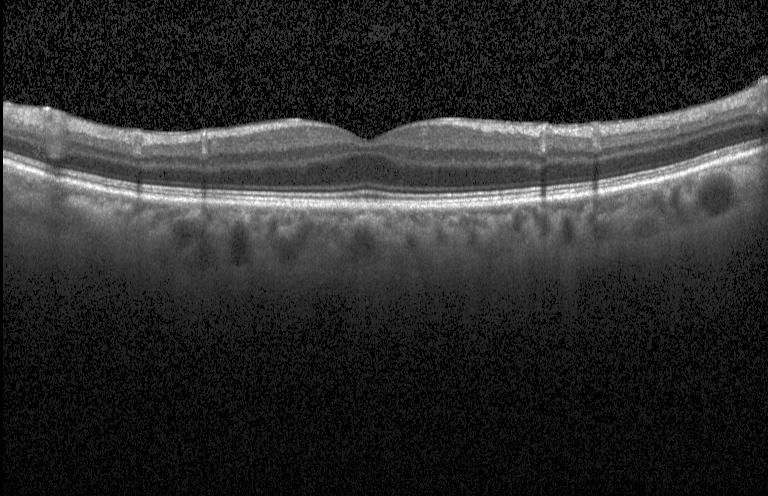
Optical coherence tomography B-scan. Impression: neither choroidal neovascularization, diabetic macular edema, nor drusen.